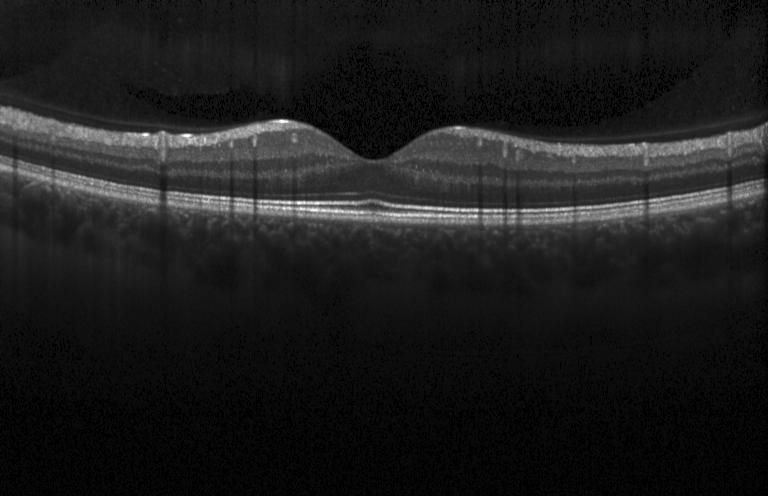
Optical coherence tomography B-scan · through the macula — Macular OCT: no evidence of choroidal neovascularization, diabetic macular edema, or drusen.